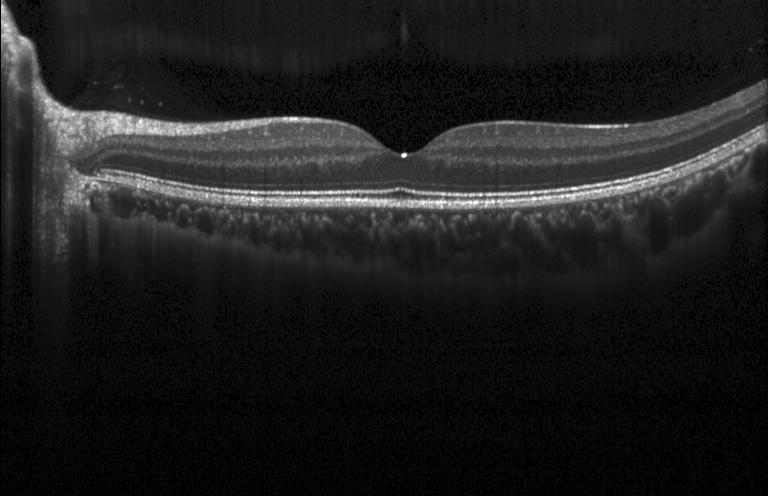

Fovea-centered · Heidelberg Spectralis · SD-OCT · retinal OCT B-scan — Diagnosis: neither CNV, DME, nor drusen.